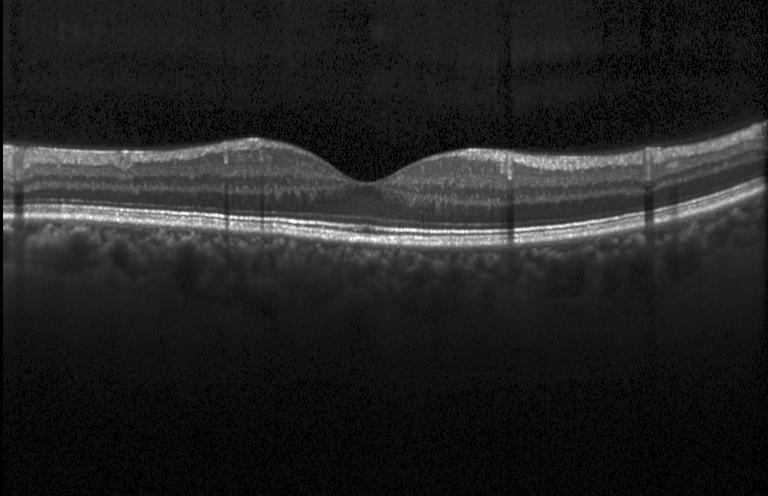
The scan shows no evidence of CNV, DME, or drusen.